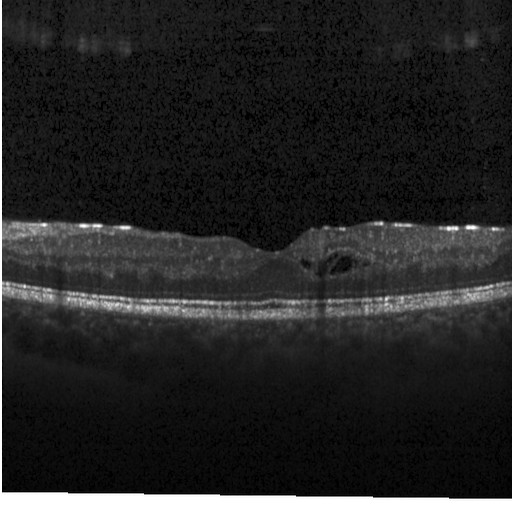
Fovea-centered; spectral-domain OCT; optical coherence tomography scan.
Diabetic macular edema.